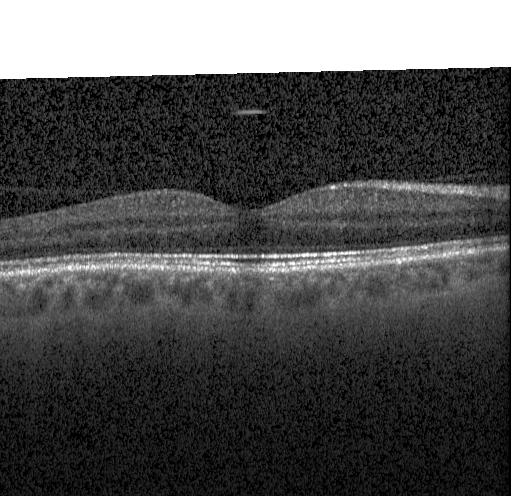
Retinal OCT cross-section
Impression: no evidence of choroidal neovascularization, diabetic macular edema, or drusen.